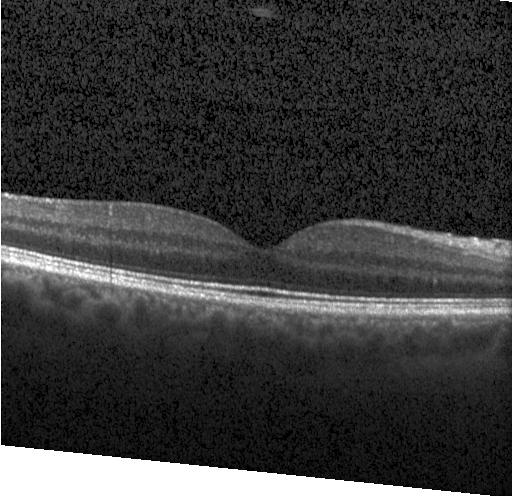
SD-OCT; through the macula; retinal OCT B-scan.
Finding: no evidence of CNV, DME, or drusen.